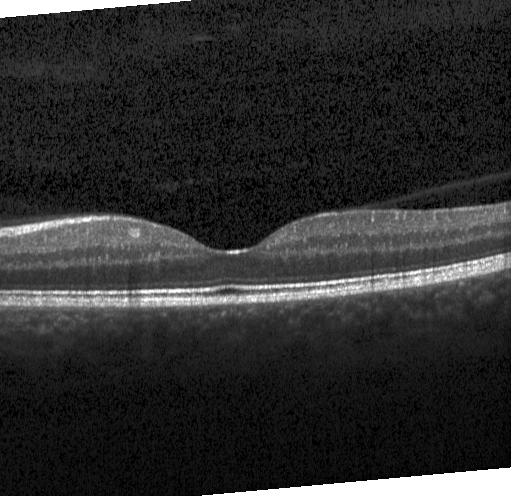

Heidelberg Spectralis · optical coherence tomography scan · spectral-domain OCT · through the macula. Impression: no evidence of CNV, DME, or drusen.